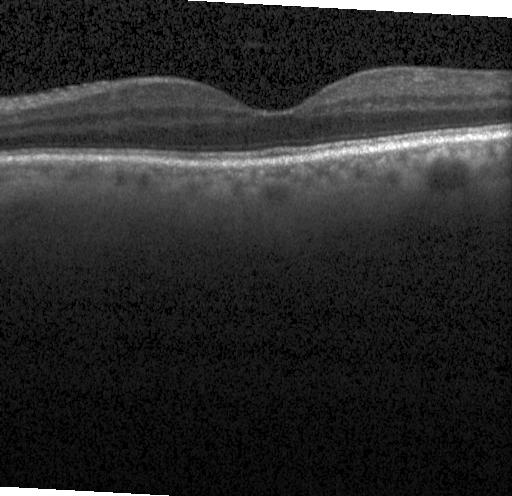

Heidelberg Spectralis; retinal OCT cross-section
Finding: neither choroidal neovascularization, diabetic macular edema, nor drusen.